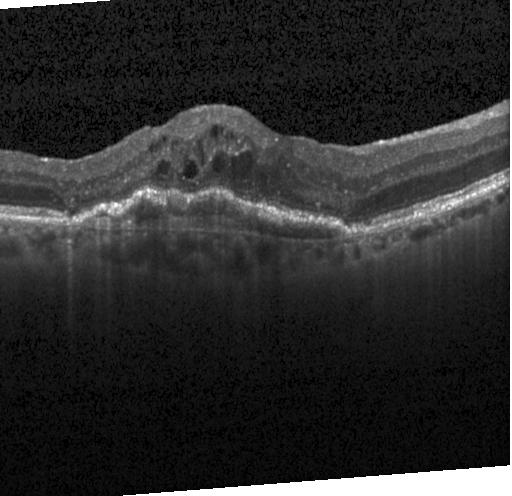
Spectral-domain OCT. Acquired on a Heidelberg Spectralis. Retinal OCT B-scan. Fovea-centered
OCT finding: a choroidal neovascular membrane.